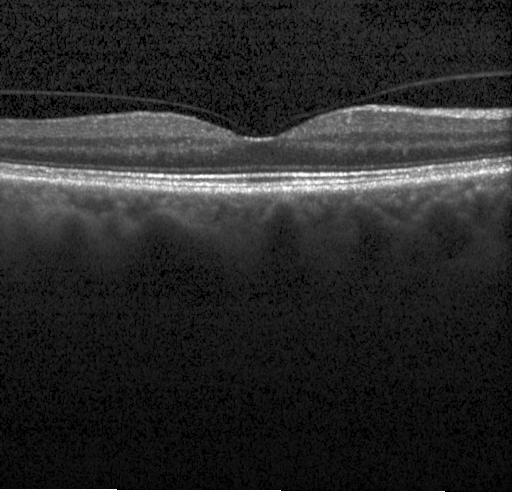 OCT line scan; spectral-domain optical coherence tomography; fovea-centered.
Finding: no choroidal neovascularization, diabetic macular edema, or drusen.